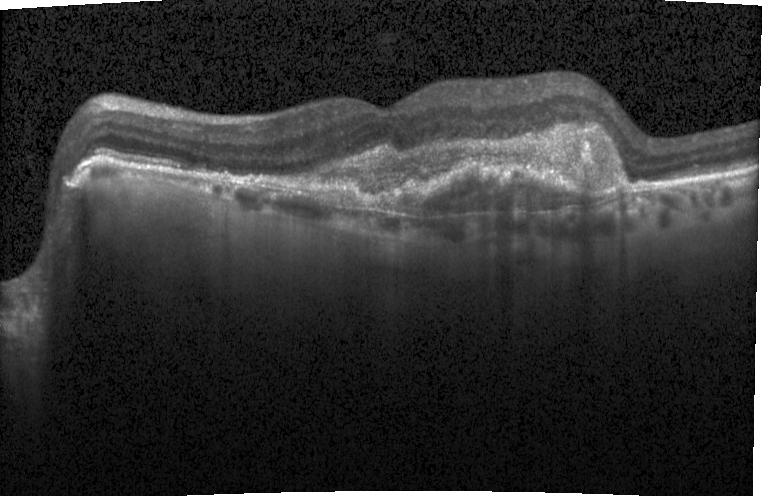

Fovea-centered. Optical coherence tomography B-scan — A choroidal neovascular membrane.